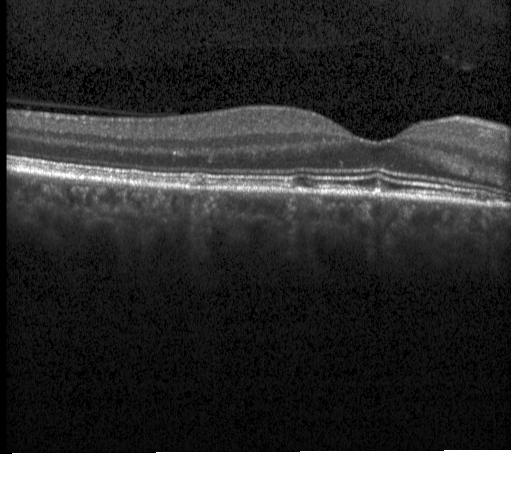 Horizontal scan through the fovea; OCT line scan; Heidelberg Spectralis; spectral-domain OCT. Drusen.